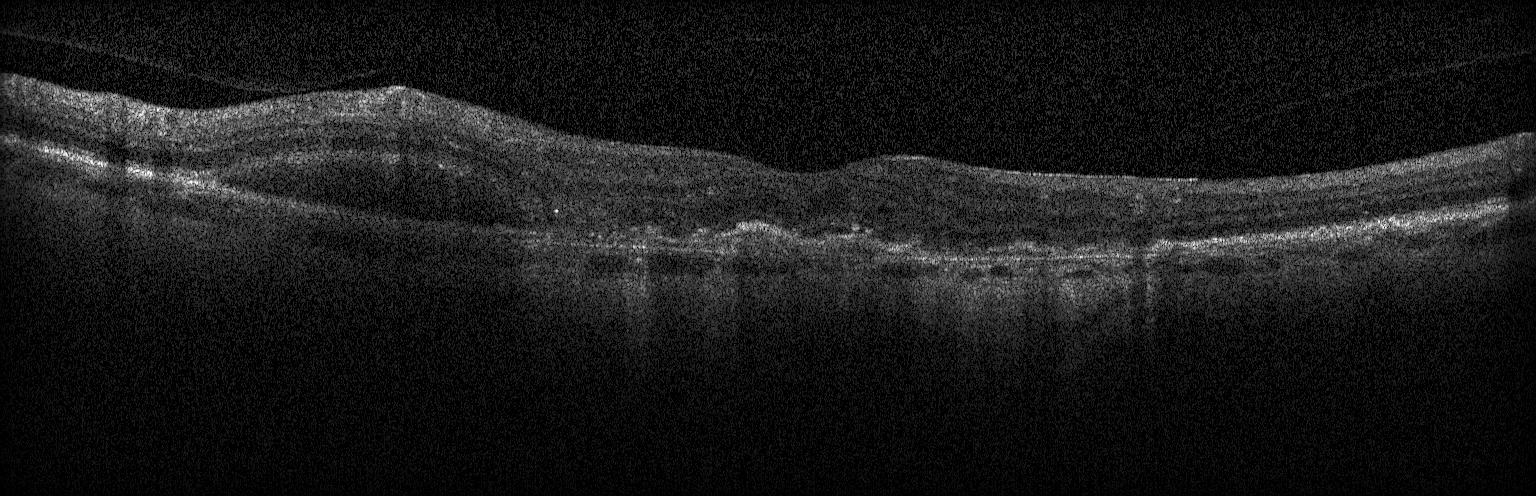 Macular OCT demonstrating CNV.